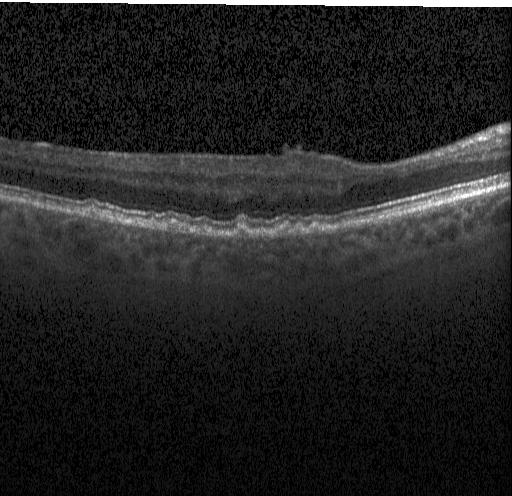

Optical coherence tomography scan. Horizontal scan through the fovea
Diagnosis: drusen.